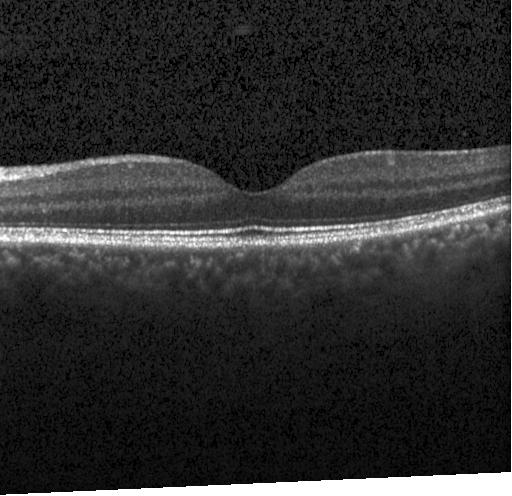

Macular OCT demonstrating no choroidal neovascularization, diabetic macular edema, or drusen.